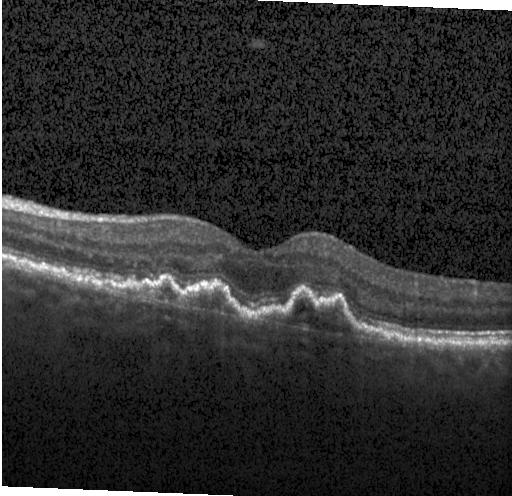
Acquired on a Heidelberg Spectralis. Retinal OCT cross-section. Centered on the fovea. OCT finding: a choroidal neovascular membrane.